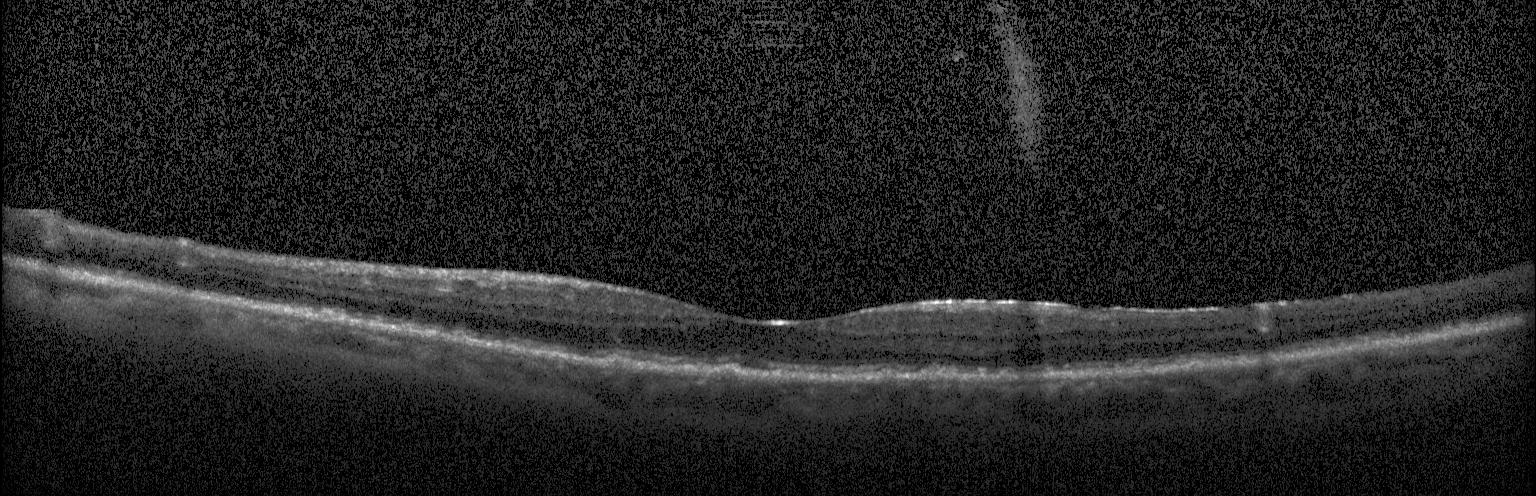
Spectral-domain OCT. Macular scan. Retinal OCT B-scan. Heidelberg Spectralis. Finding: drusen.